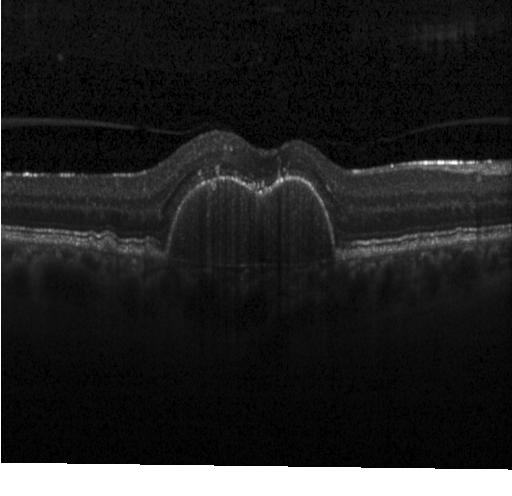 Acquired on a Heidelberg Spectralis; through the macula; spectral-domain OCT; retinal OCT B-scan — OCT finding: a choroidal neovascular membrane.